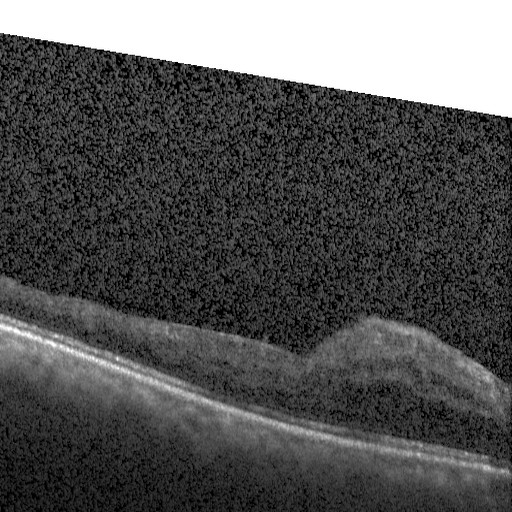 Retinal OCT cross-section, centered on the fovea. This B-scan demonstrates DME.